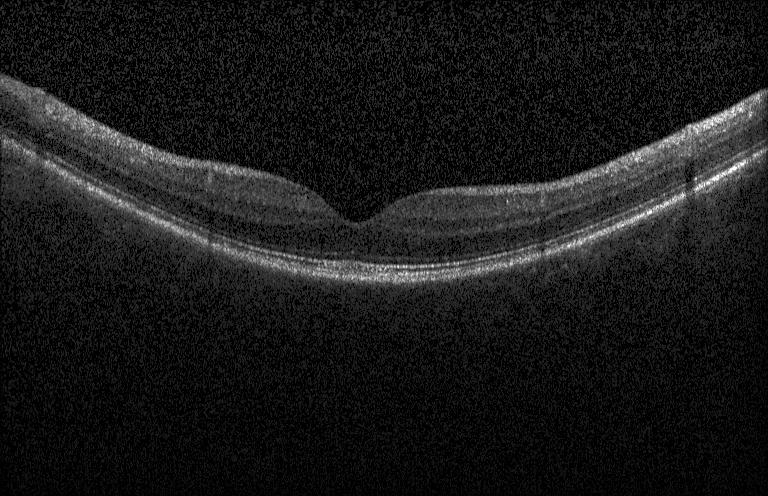

Retinal OCT B-scan
Diagnosis: no CNV, no DME, and no drusen.